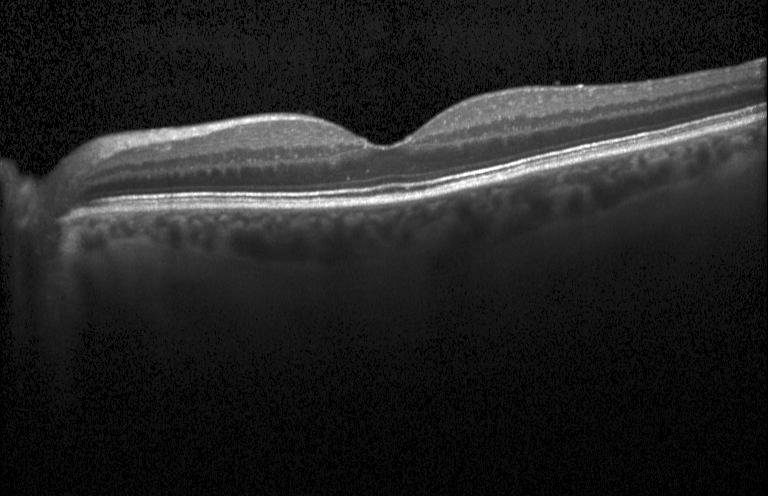

Acquired on a Heidelberg Spectralis. Spectral-domain OCT. Retinal OCT cross-section
Diagnosis: no evidence of choroidal neovascularization, diabetic macular edema, or drusen.